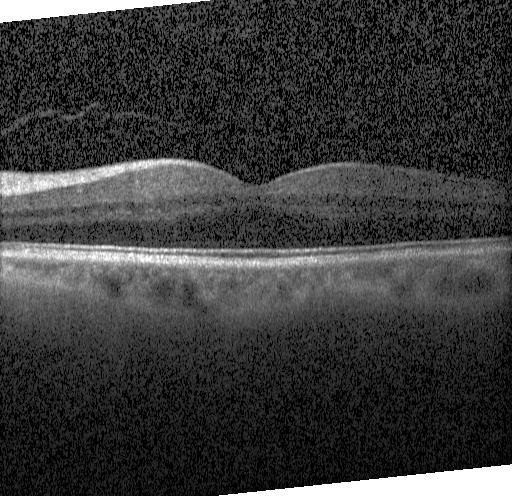
This B-scan demonstrates no choroidal neovascularization, no diabetic macular edema, and no drusen.